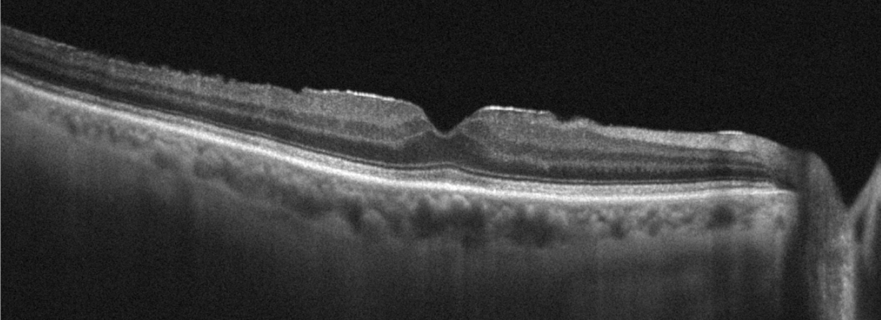 Impression: epiretinal membrane.